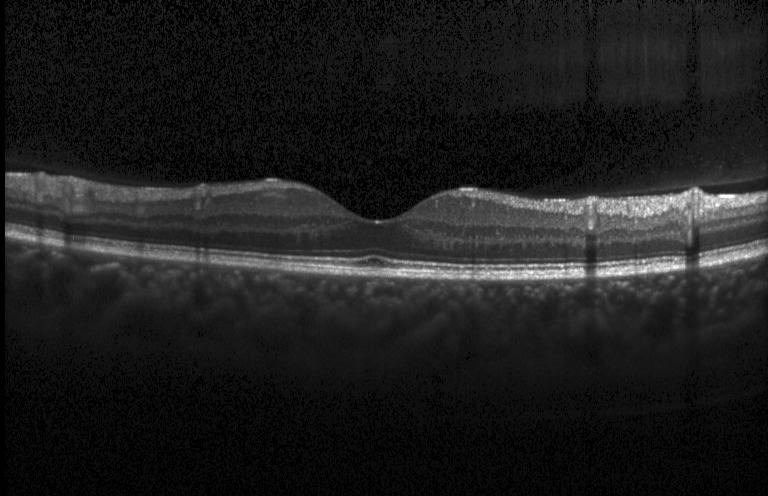

The scan shows neither choroidal neovascularization, diabetic macular edema, nor drusen.